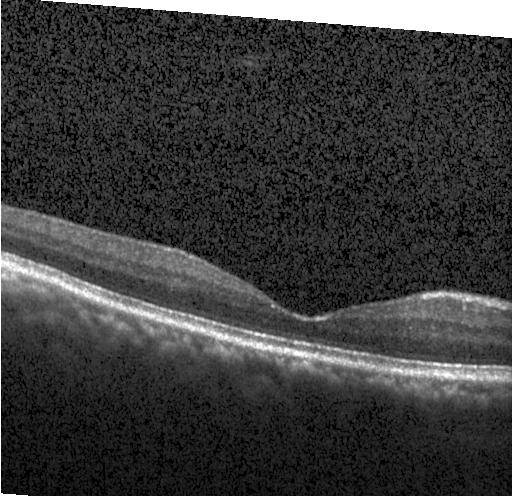

Retinal OCT cross-section.
Finding: neither CNV, DME, nor drusen.